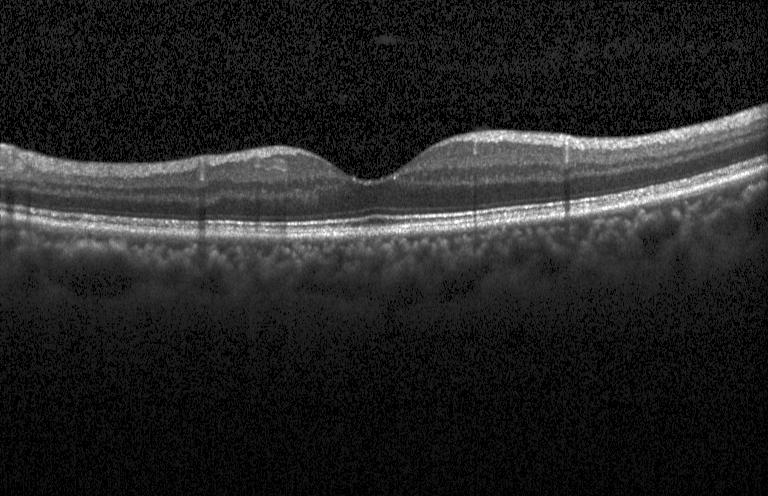
Dx: no evidence of choroidal neovascularization, diabetic macular edema, or drusen.